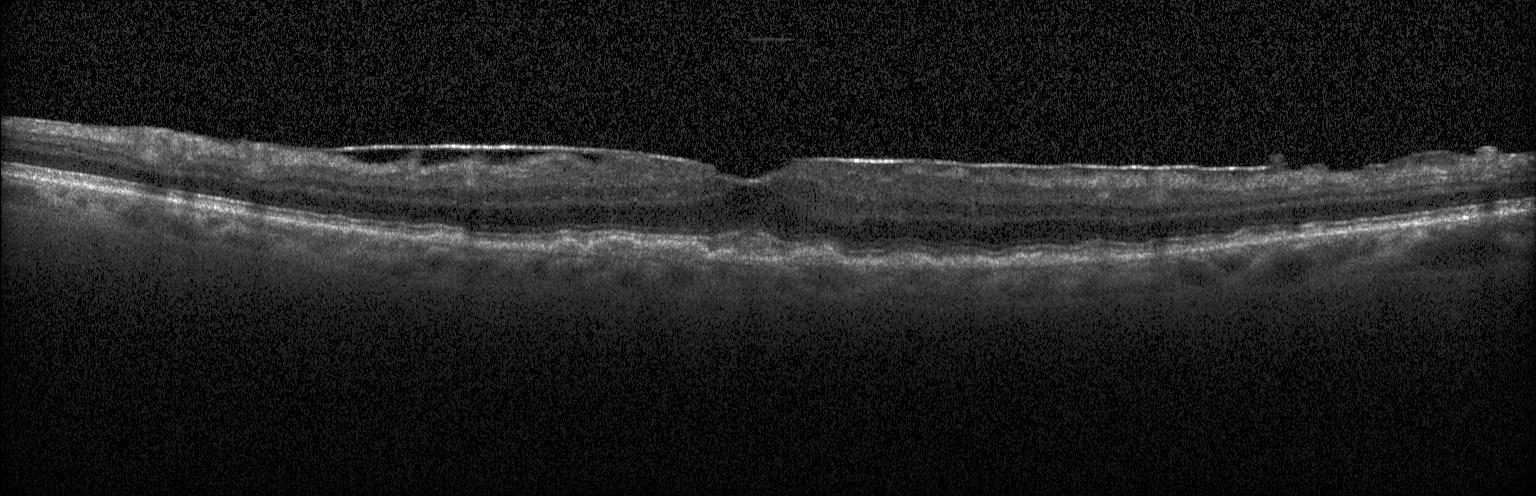

OCT line scan — Diagnosis: multiple drusen.